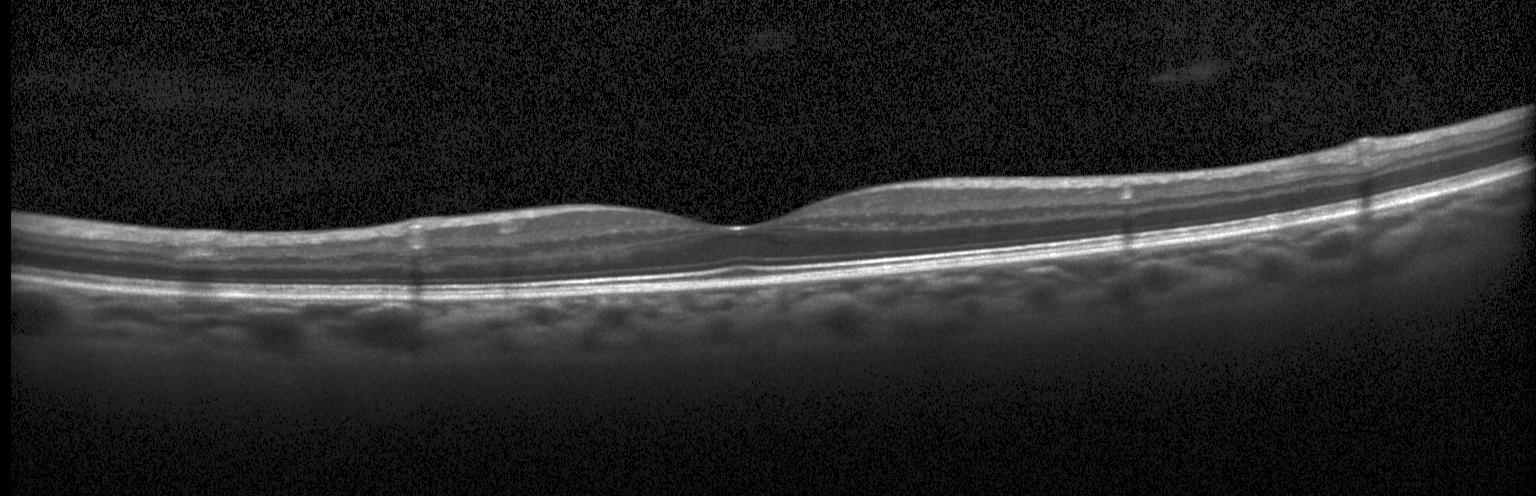
The scan shows neither CNV, DME, nor drusen.